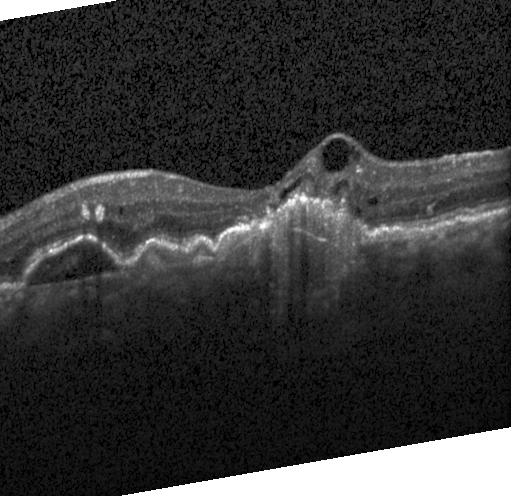

Instrument: Heidelberg Spectralis. Spectral-domain OCT. OCT line scan. Macular scan — Assessment: a choroidal neovascular membrane.